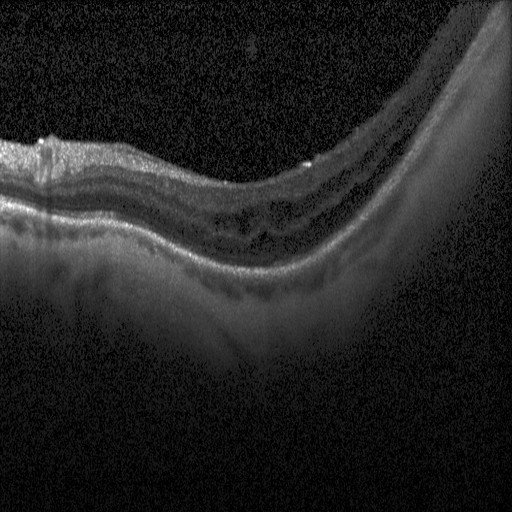 Diagnosis: diabetic macular edema.